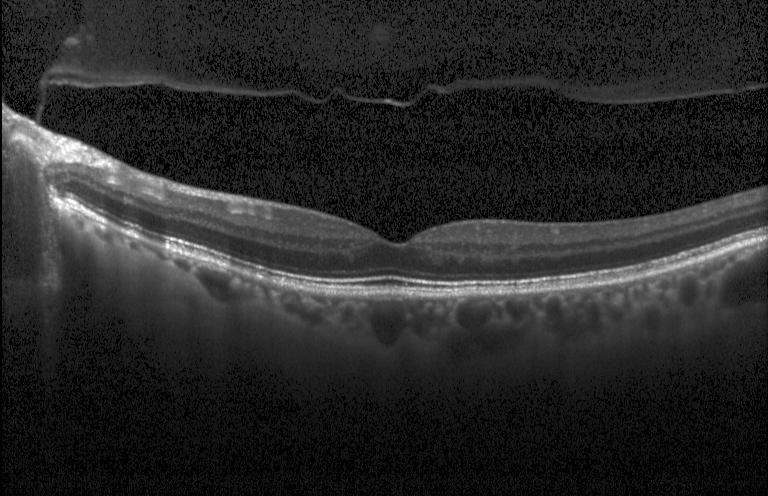 Spectral-domain OCT · OCT B-scan · horizontal scan through the fovea · Heidelberg Spectralis — Impression: neither choroidal neovascularization, diabetic macular edema, nor drusen.